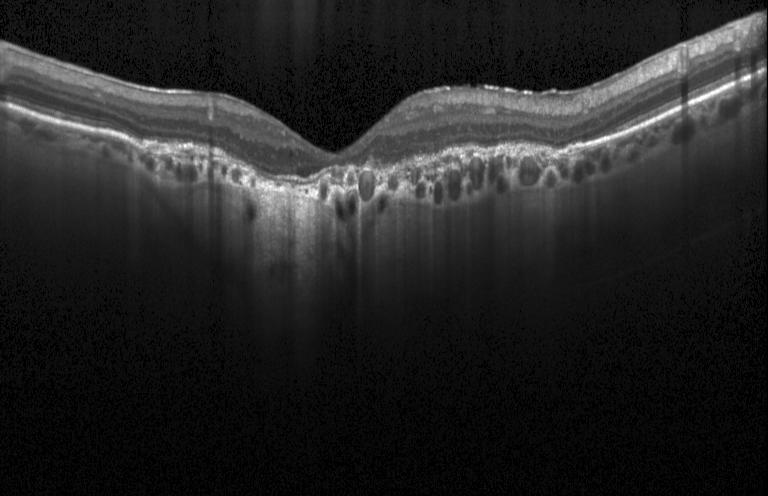

Finding: a choroidal neovascular membrane.